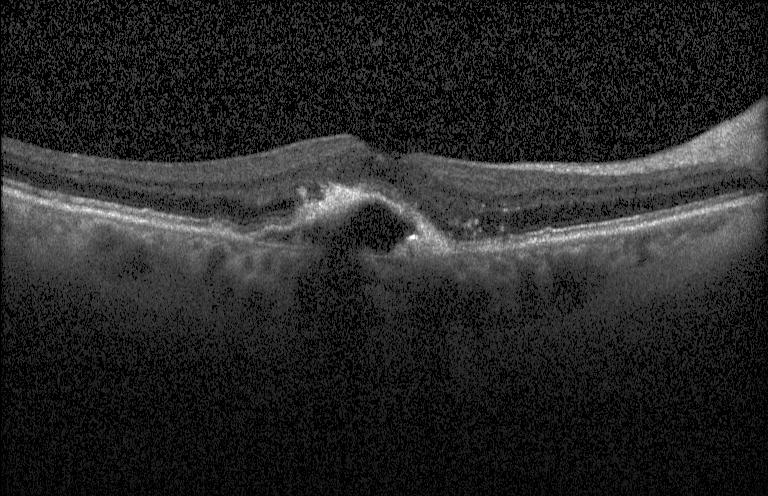

Impression: a choroidal neovascular membrane.